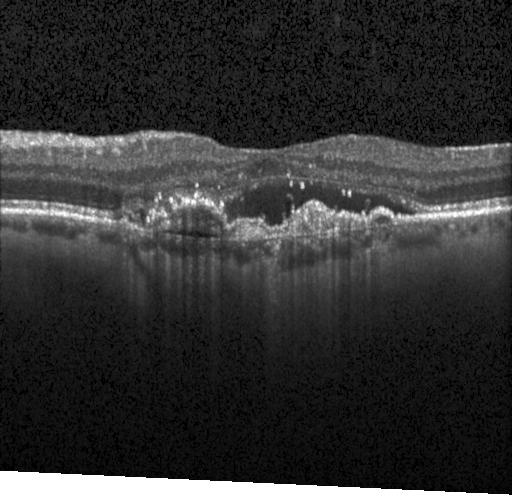 Finding: CNV.